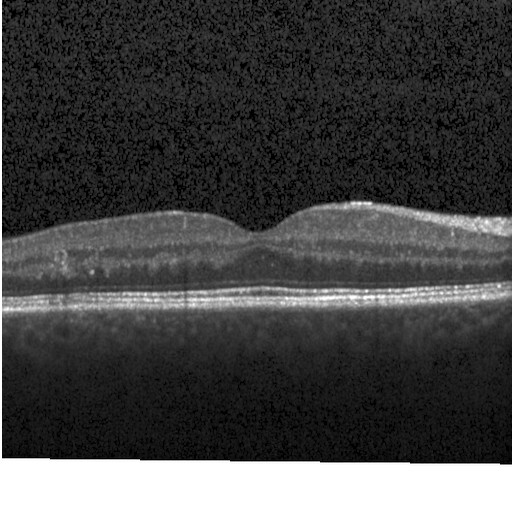
Heidelberg Spectralis OCT system; spectral-domain OCT; optical coherence tomography scan; centered on the fovea — Impression: diabetic macular edema (DME).